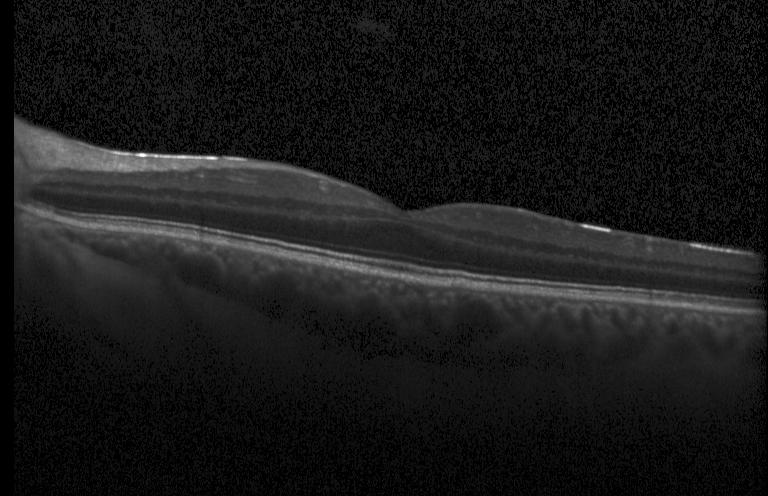

This B-scan demonstrates no evidence of choroidal neovascularization, diabetic macular edema, or drusen.